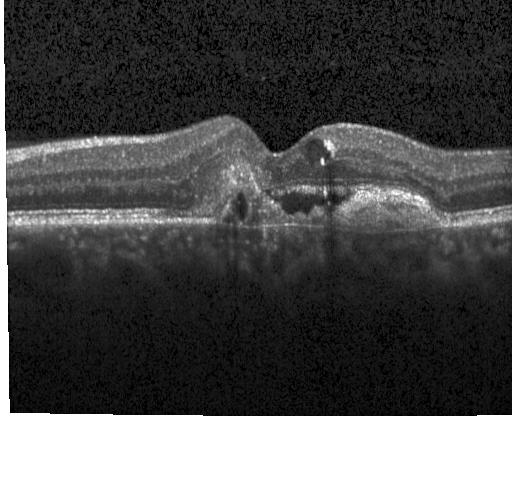

Instrument: Heidelberg Spectralis; fovea-centered; optical coherence tomography scan
Finding: a choroidal neovascular membrane.